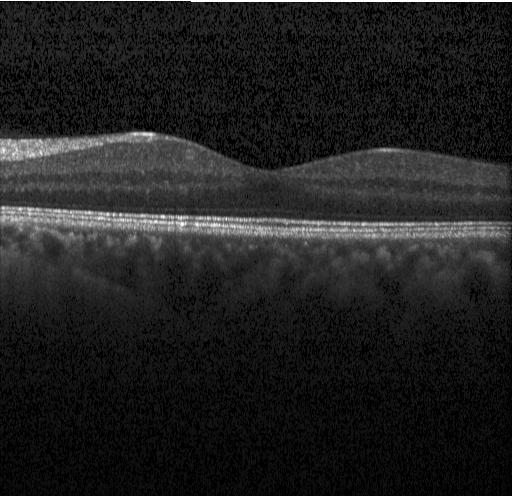
Macular scan · OCT B-scan · spectral-domain optical coherence tomography.
Finding: no evidence of CNV, DME, or drusen.